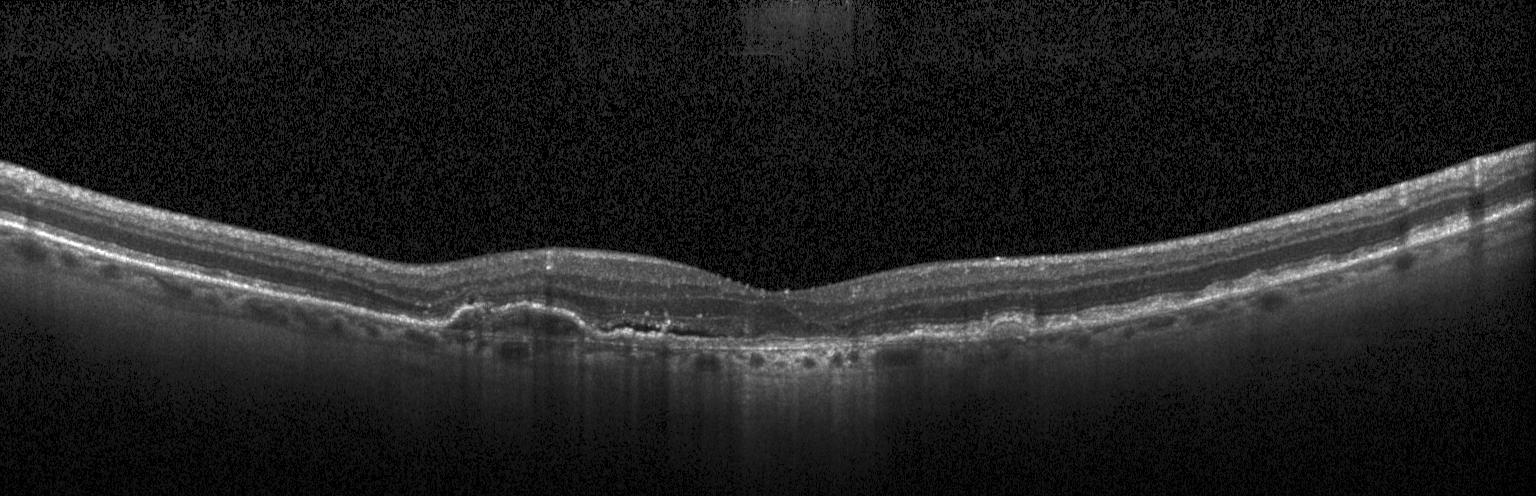 OCT B-scan. Finding: a choroidal neovascular membrane.